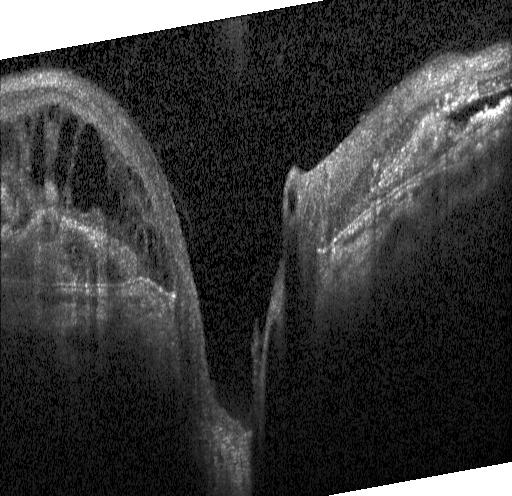

Impression: CNV.